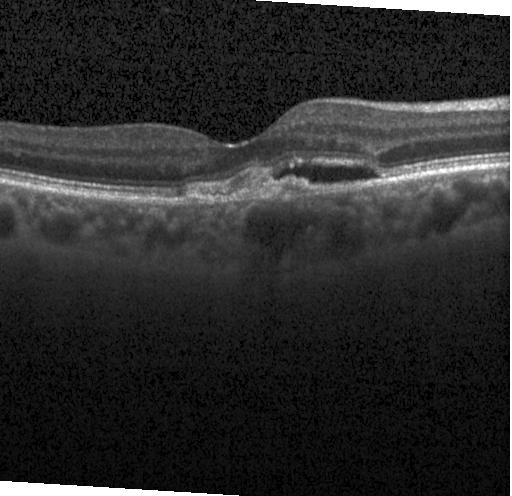 Impression: a choroidal neovascular membrane.